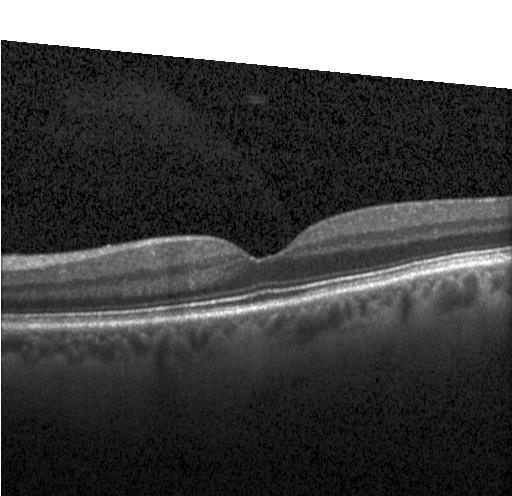
Finding: neither choroidal neovascularization, diabetic macular edema, nor drusen.